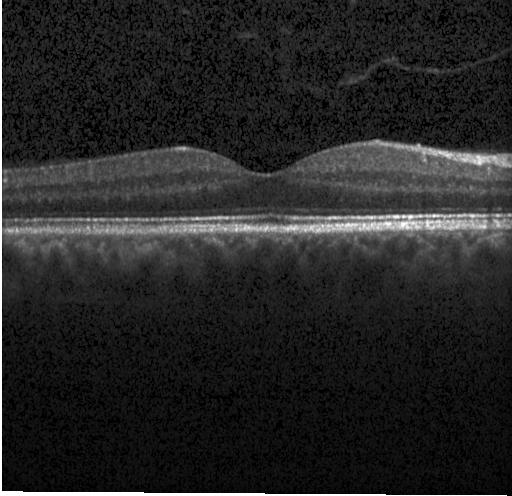 Centered on the fovea. Retinal OCT B-scan. SD-OCT. Instrument: Heidelberg Spectralis.
This B-scan demonstrates no choroidal neovascularization, diabetic macular edema, or drusen.